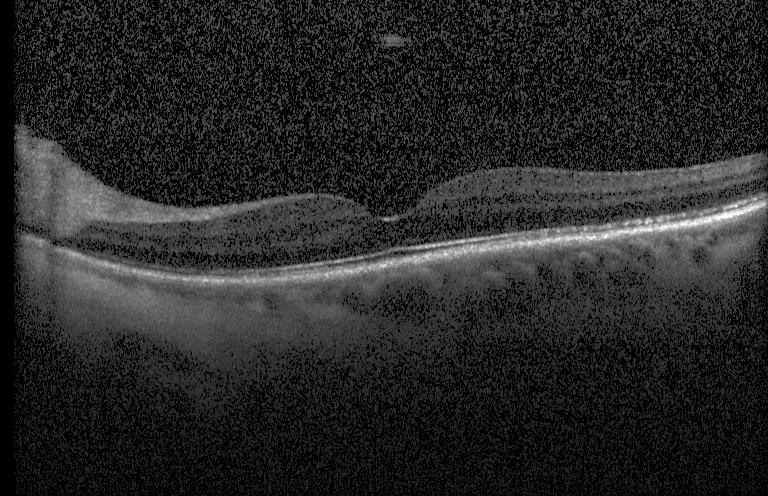 Dx: no evidence of CNV, DME, or drusen.